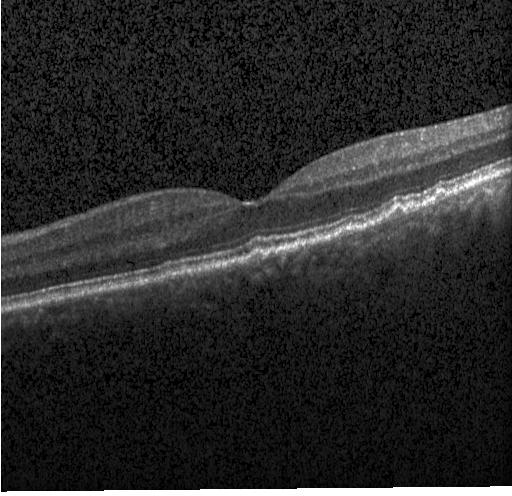 Retinal OCT cross-section showing drusen.